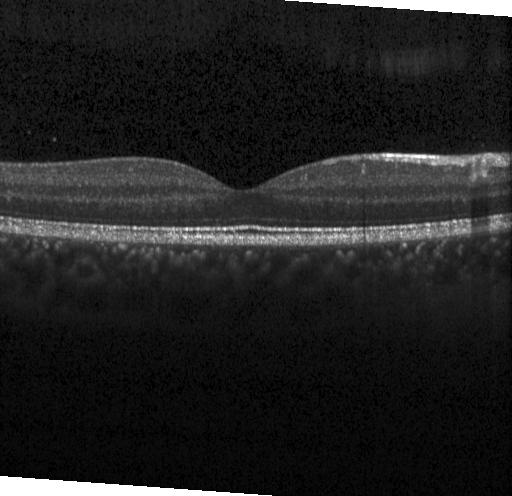
Assessment: no evidence of choroidal neovascularization, diabetic macular edema, or drusen.